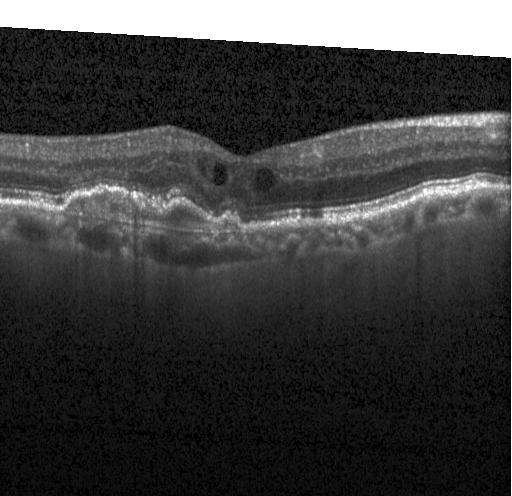 This B-scan demonstrates a choroidal neovascular membrane.